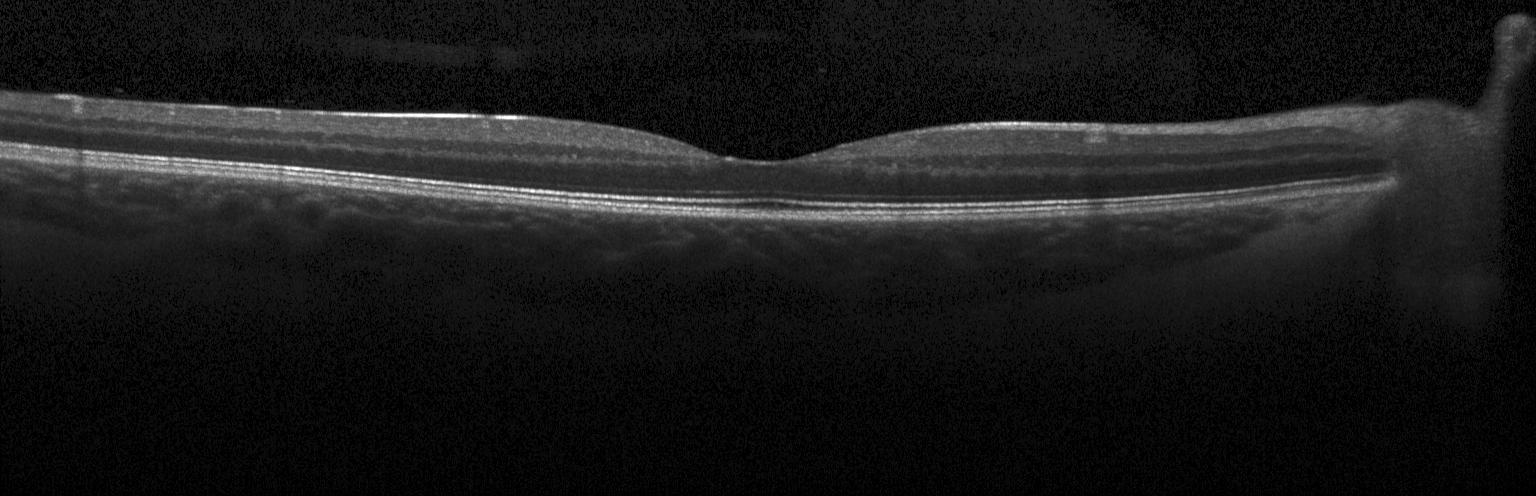 Instrument: Heidelberg Spectralis · retinal OCT B-scan
This B-scan demonstrates neither CNV, DME, nor drusen.